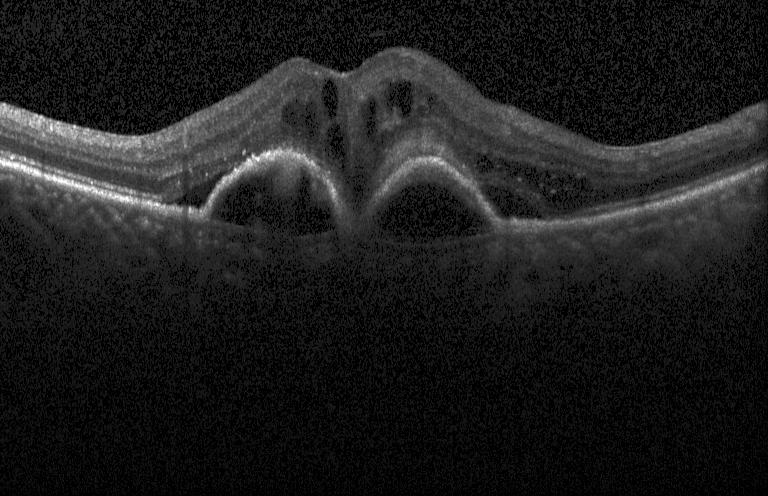 OCT B-scan showing a choroidal neovascular membrane.